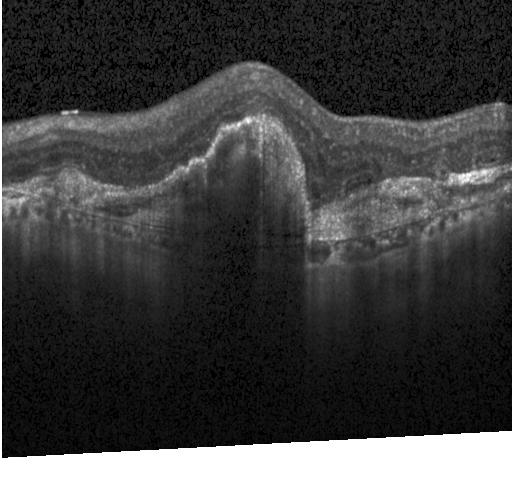 Spectral-domain OCT B-scan: a choroidal neovascular membrane.